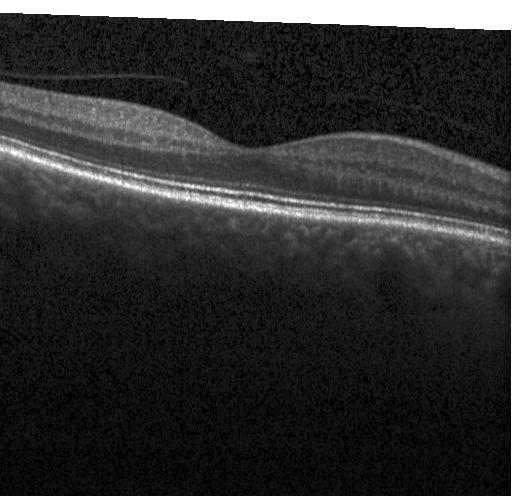

SD-OCT, instrument: Heidelberg Spectralis, retinal OCT cross-section, fovea-centered — Impression: no choroidal neovascularization, diabetic macular edema, or drusen.